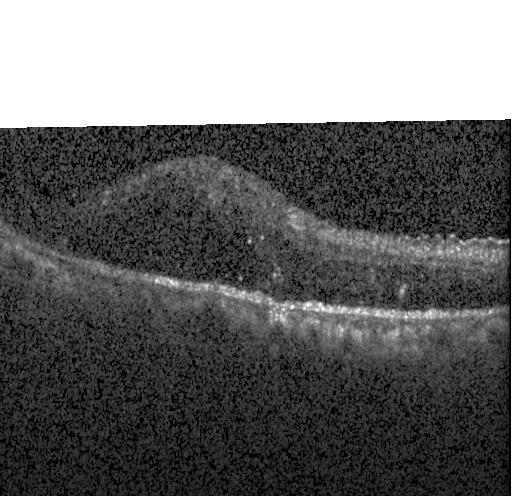

Macular scan. Spectral-domain OCT. Optical coherence tomography B-scan. Instrument: Heidelberg Spectralis.
This B-scan demonstrates diabetic macular edema (DME).